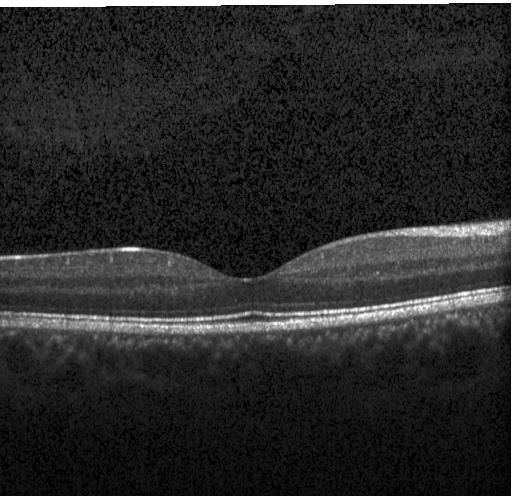
Retinal OCT cross-section showing no CNV, no DME, and no drusen.